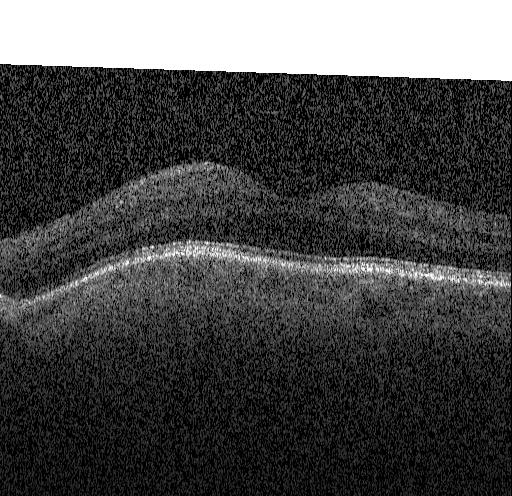
Retinal OCT B-scan; Heidelberg Spectralis; horizontal scan through the fovea; spectral-domain OCT. OCT finding: no evidence of choroidal neovascularization, diabetic macular edema, or drusen.